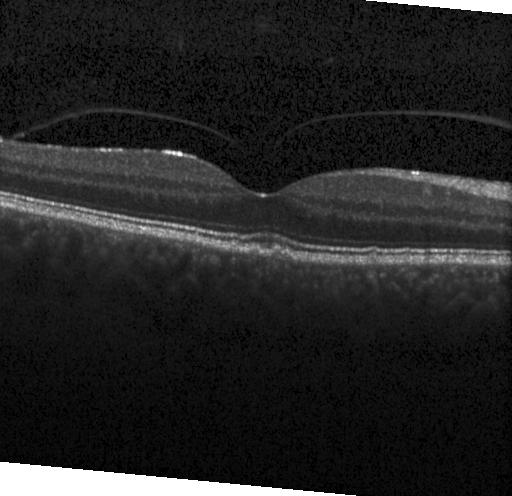
Macular OCT demonstrating multiple drusen.